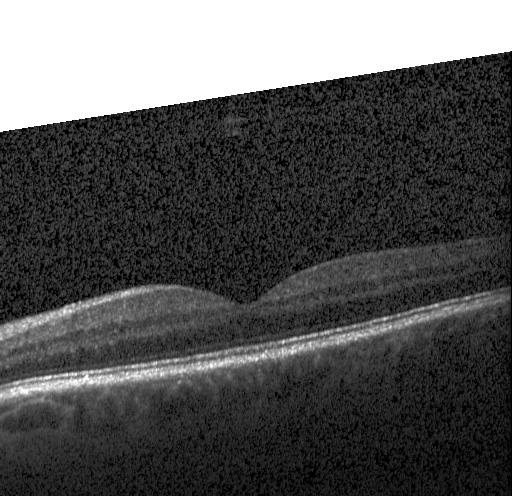 OCT scan showing no CNV, DME, or drusen.